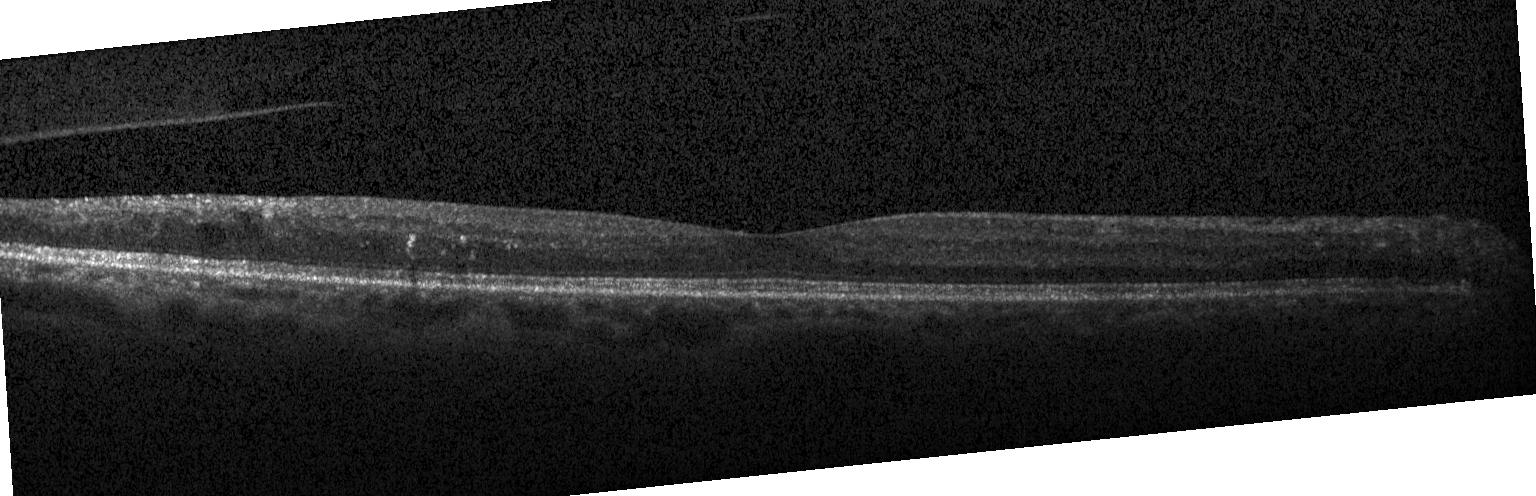 This B-scan demonstrates diabetic macular edema (DME).